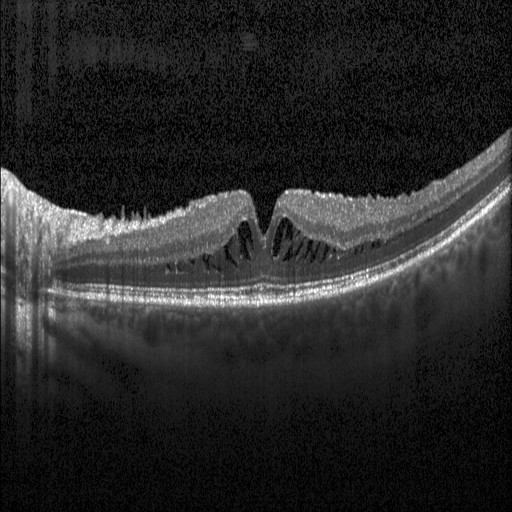 Optical coherence tomography scan · spectral-domain optical coherence tomography — The scan shows DME.